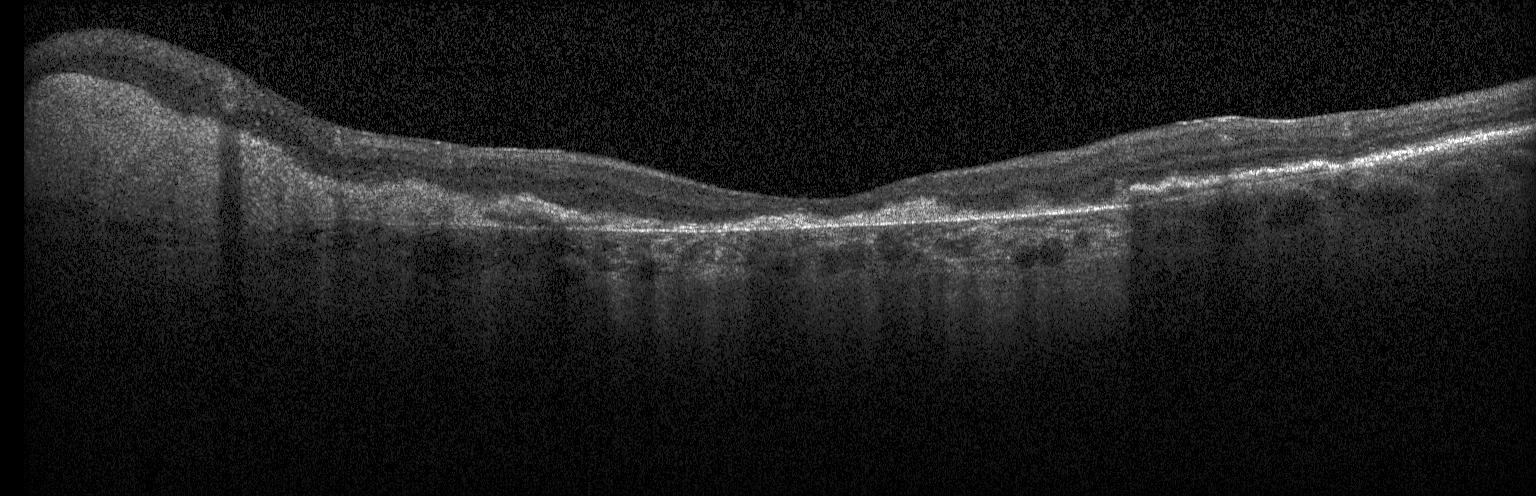
Through the macula, optical coherence tomography scan, instrument: Heidelberg Spectralis — OCT finding: choroidal neovascularization (CNV).